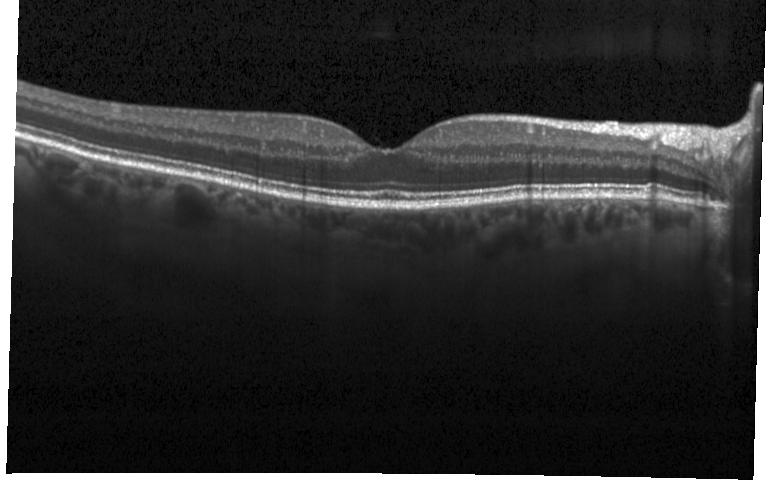

No CNV, no DME, and no drusen.